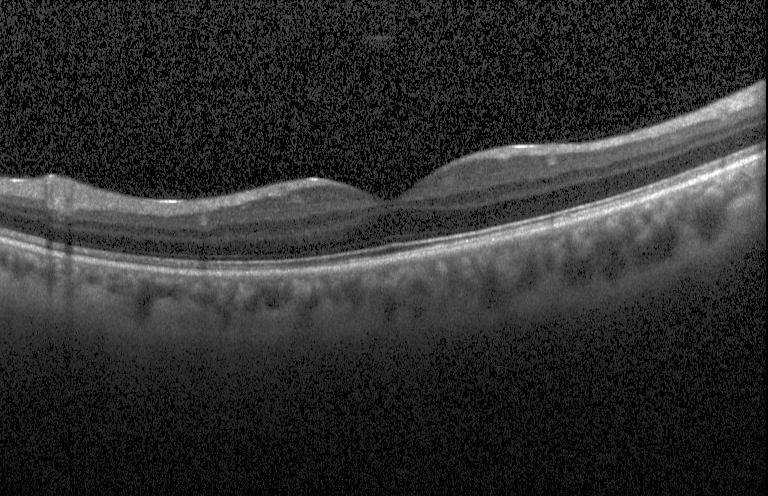

Acquired on a Heidelberg Spectralis. Spectral-domain OCT. Retinal OCT cross-section.
No CNV, DME, or drusen.